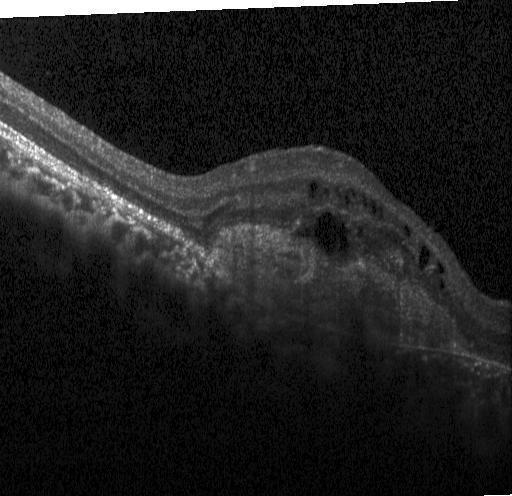 Assessment: a choroidal neovascular membrane.